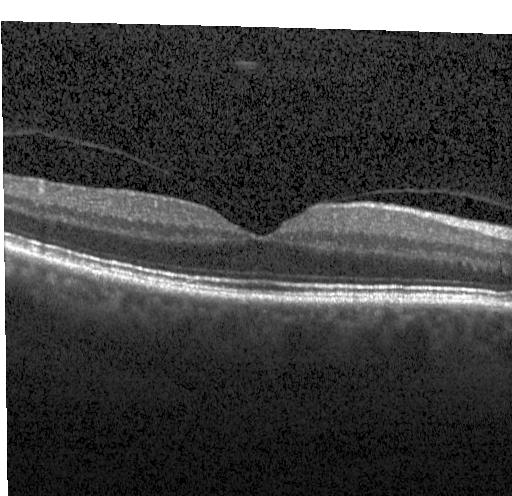

Heidelberg Spectralis OCT system. Optical coherence tomography scan. Centered on the fovea. Macular OCT: no evidence of choroidal neovascularization, diabetic macular edema, or drusen.